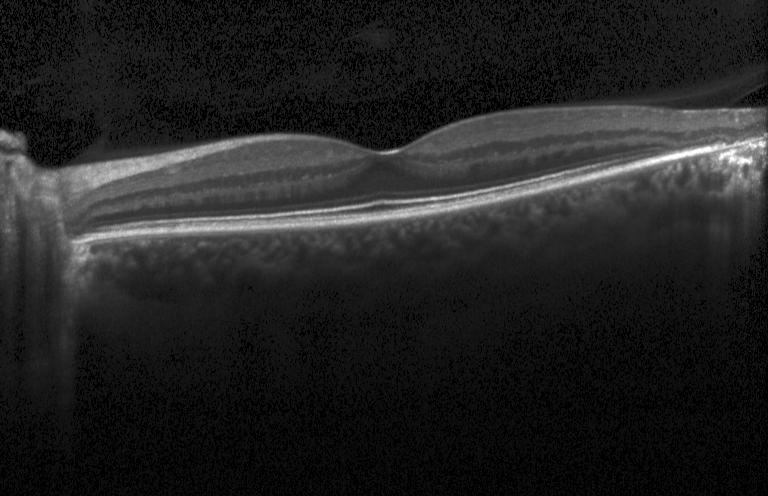 Diagnosis: neither choroidal neovascularization, diabetic macular edema, nor drusen.